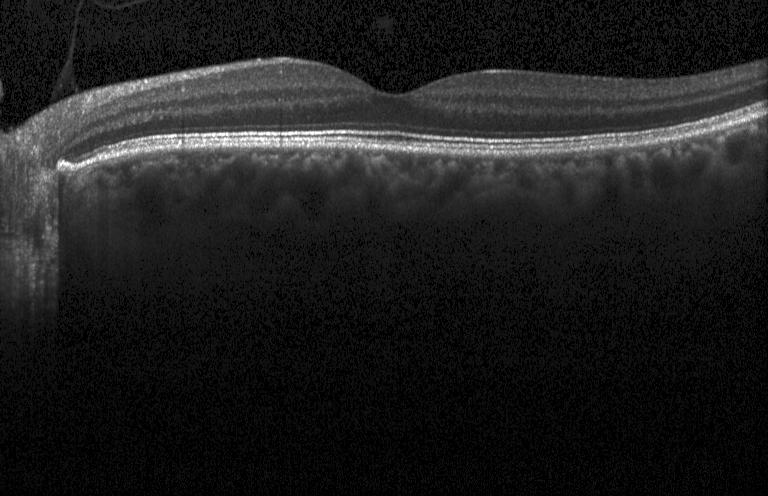

Centered on the fovea; instrument: Heidelberg Spectralis; spectral-domain OCT; OCT B-scan. Assessment: no evidence of CNV, DME, or drusen.